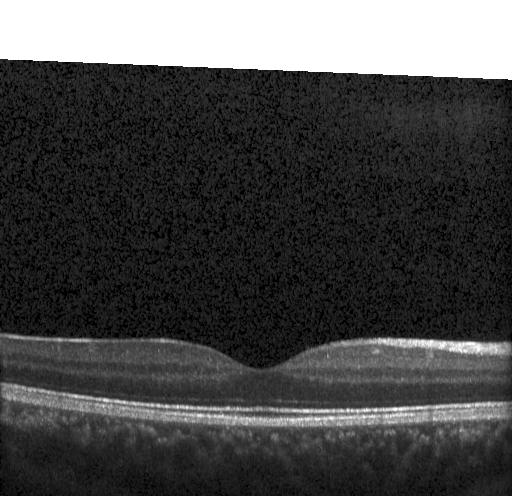 OCT scan showing neither choroidal neovascularization, diabetic macular edema, nor drusen.